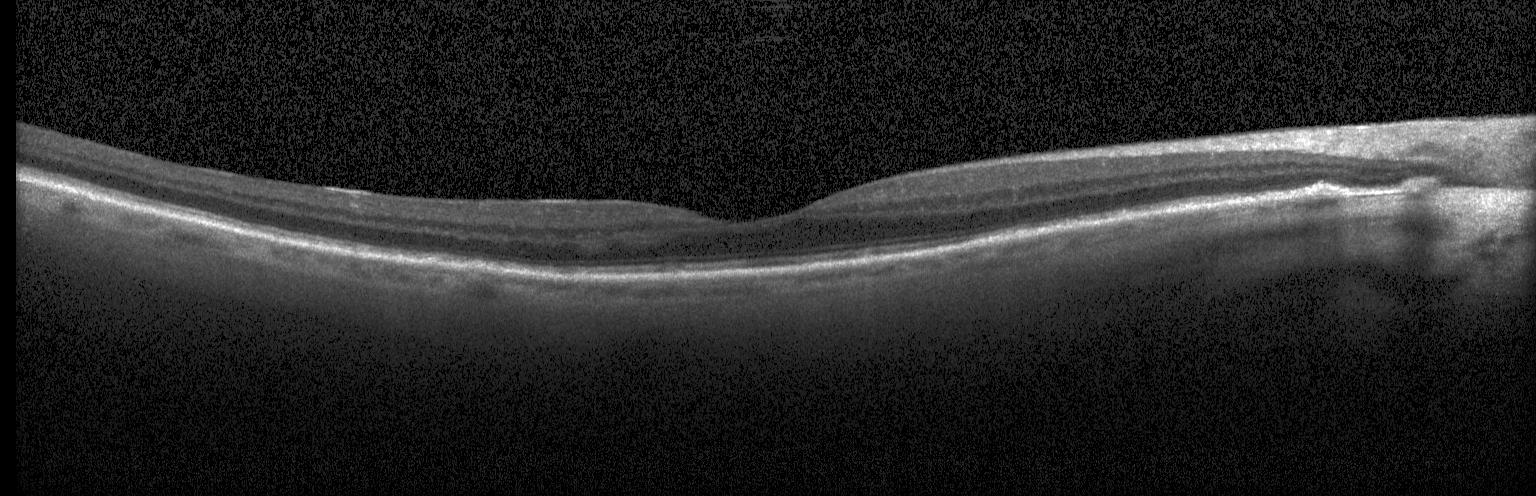
OCT scan showing neither choroidal neovascularization, diabetic macular edema, nor drusen.